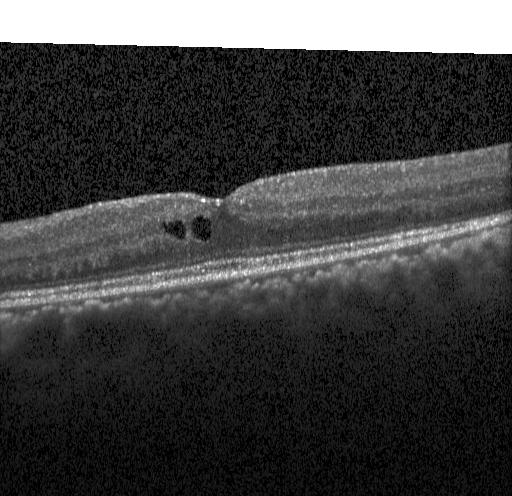
Optical coherence tomography B-scan. Spectral-domain optical coherence tomography. Acquired on a Heidelberg Spectralis. Horizontal scan through the fovea. Finding: diabetic macular edema (DME).